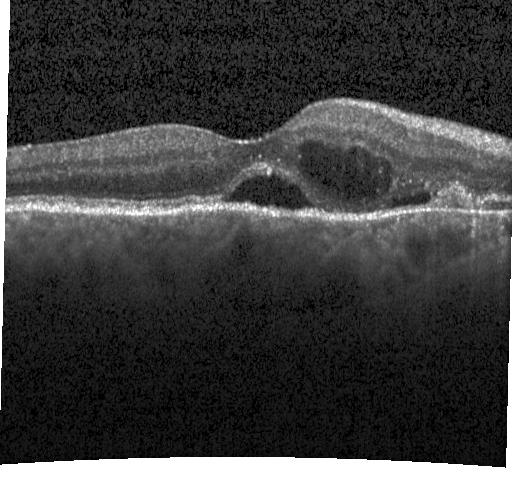

Through the macula · instrument: Heidelberg Spectralis · retinal OCT B-scan. Finding: choroidal neovascularization.